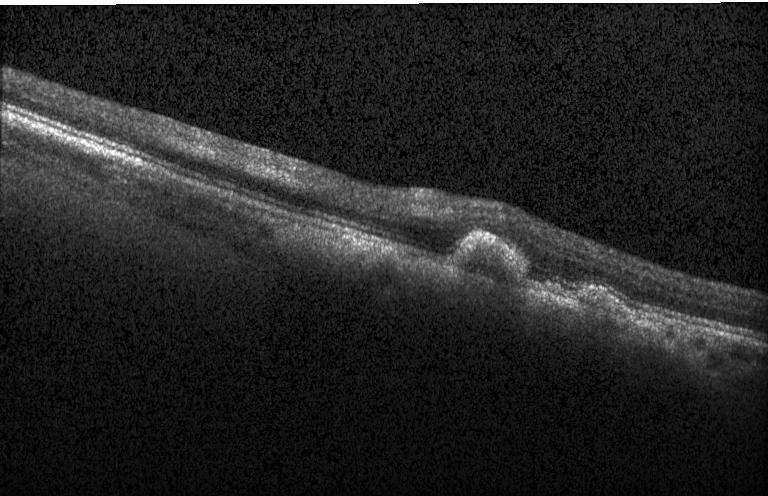

Finding: a choroidal neovascular membrane.